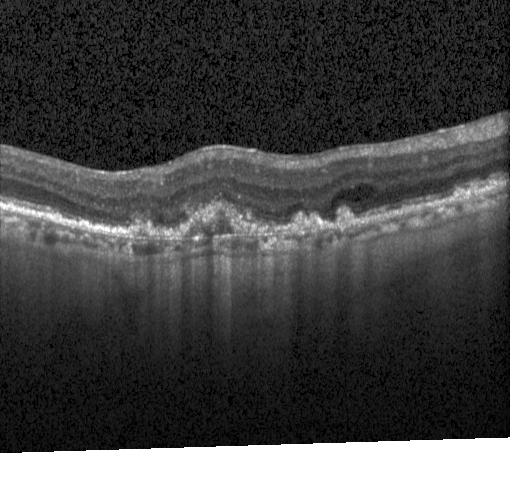 Fovea-centered; spectral-domain optical coherence tomography; retinal OCT B-scan — Impression: a choroidal neovascular membrane.